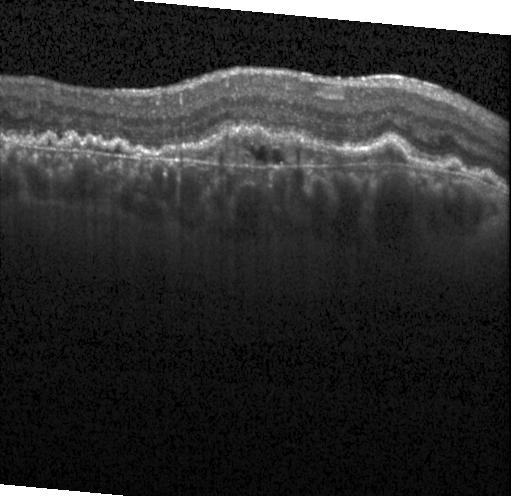 OCT line scan · acquired on a Heidelberg Spectralis — Finding: a choroidal neovascular membrane.